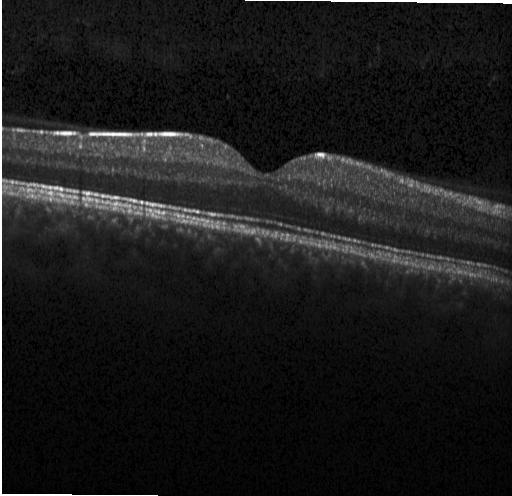
Horizontal scan through the fovea; Heidelberg Spectralis; optical coherence tomography scan.
The scan shows no evidence of choroidal neovascularization, diabetic macular edema, or drusen.